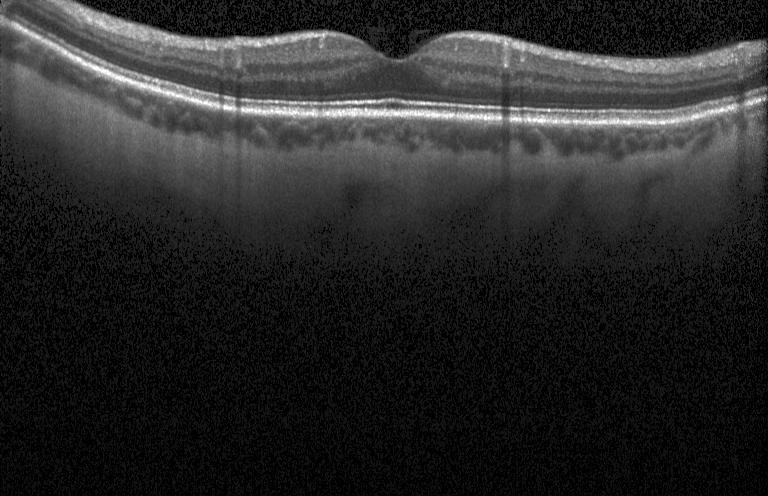
Macular scan. Optical coherence tomography scan. Heidelberg Spectralis
Impression: no evidence of choroidal neovascularization, diabetic macular edema, or drusen.